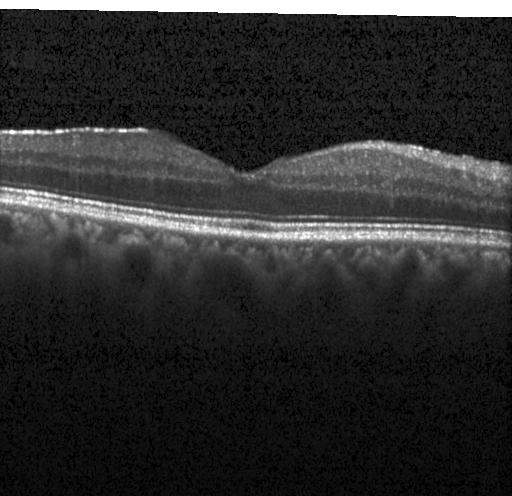
Diagnosis: no evidence of choroidal neovascularization, diabetic macular edema, or drusen.